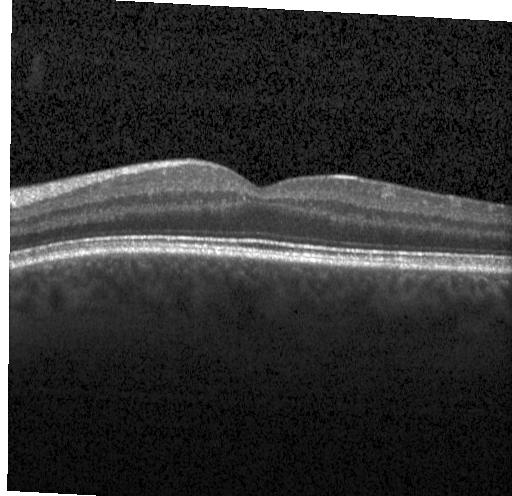

Dx: neither choroidal neovascularization, diabetic macular edema, nor drusen.